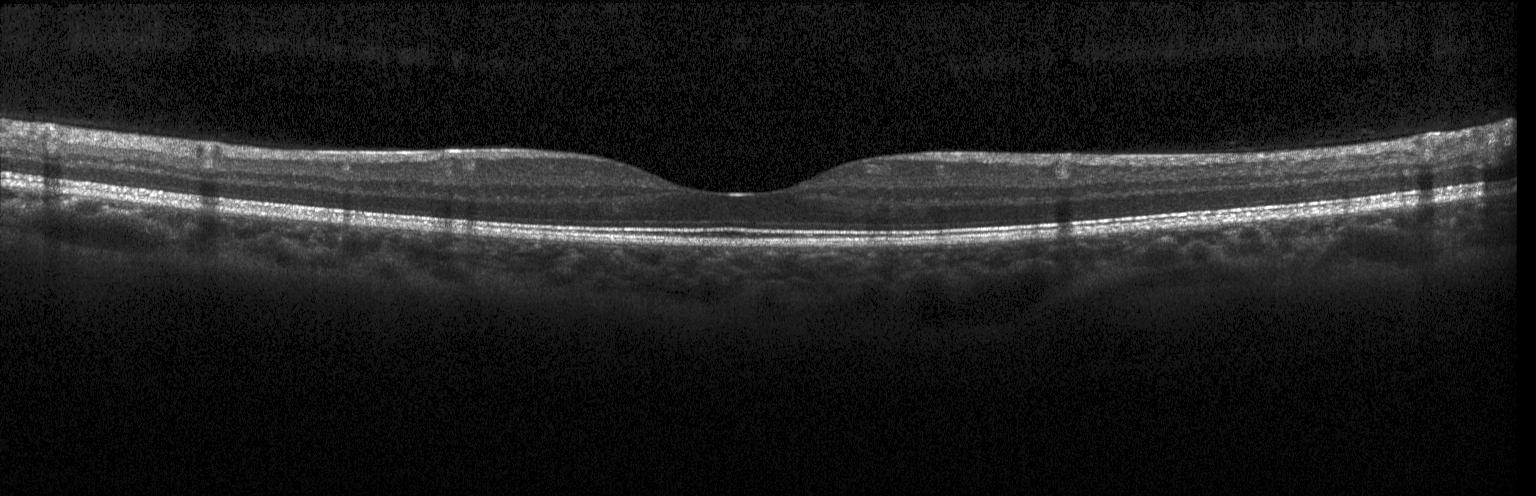

Spectral-domain OCT, retinal OCT cross-section
The scan shows neither CNV, DME, nor drusen.